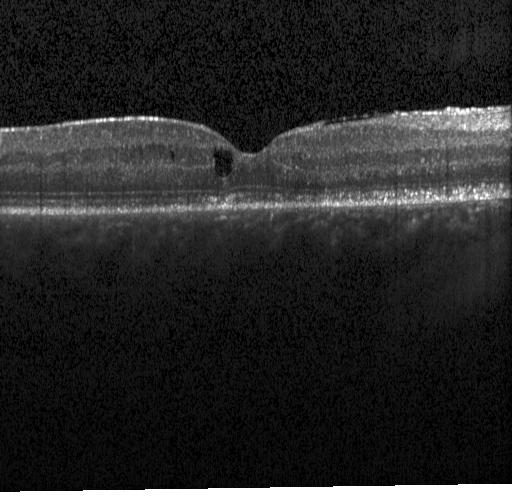 Retinal OCT cross-section, spectral-domain OCT, macular scan. Dx: diabetic macular edema (DME).